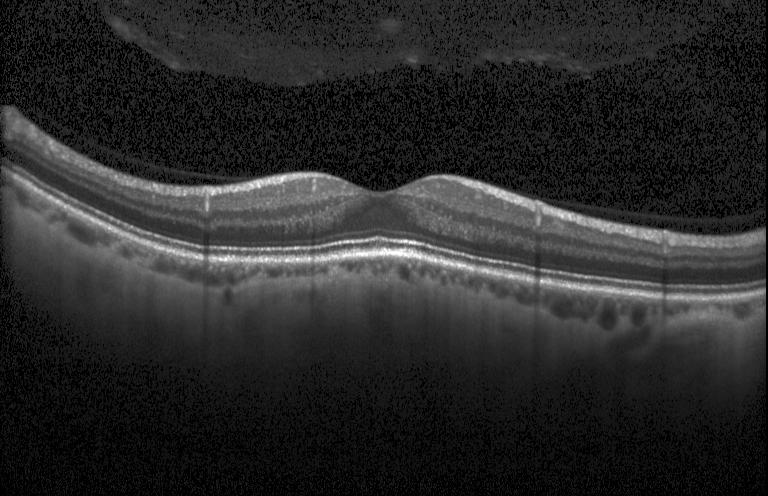 Spectral-domain optical coherence tomography, Heidelberg Spectralis OCT system, OCT line scan, through the macula — Finding: no choroidal neovascularization, diabetic macular edema, or drusen.